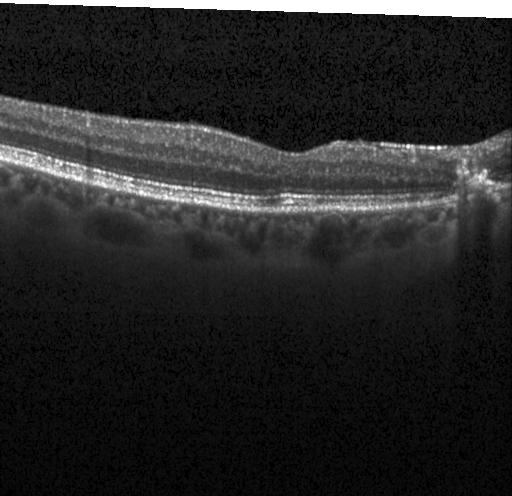 Heidelberg Spectralis · OCT B-scan. Finding: choroidal neovascularization (CNV).